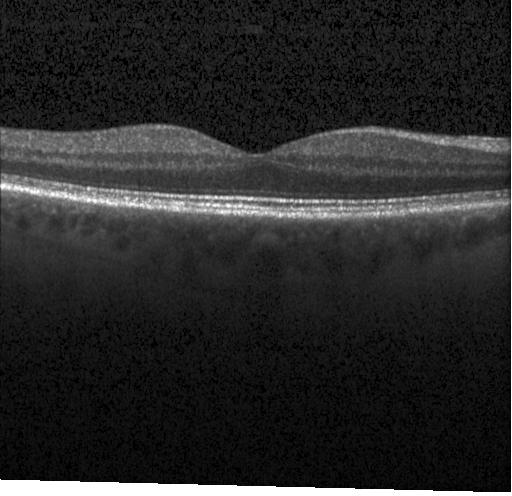

OCT B-scan. Heidelberg Spectralis
Macular OCT: neither choroidal neovascularization, diabetic macular edema, nor drusen.